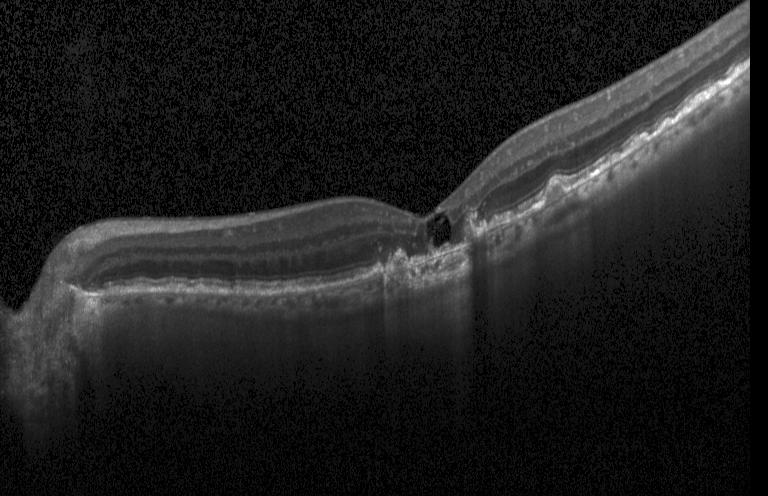

Spectral-domain OCT. Heidelberg Spectralis. Retinal OCT B-scan.
This B-scan demonstrates CNV.